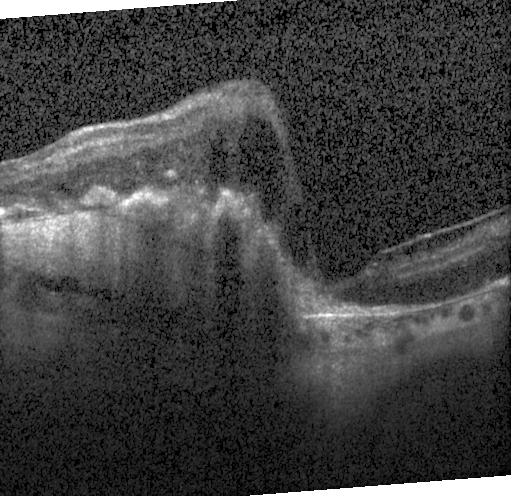
Spectral-domain OCT, optical coherence tomography B-scan — The scan shows choroidal neovascularization (CNV).